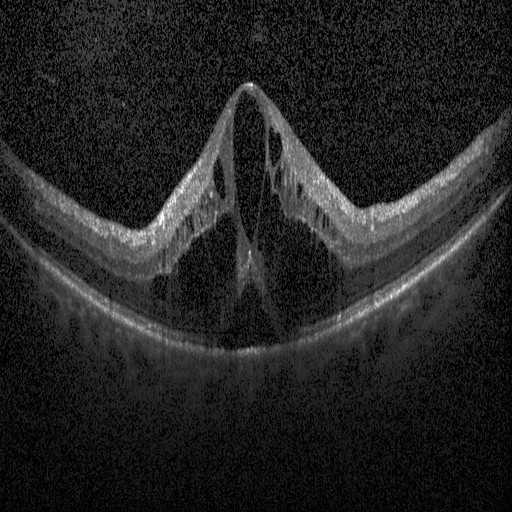 Finding: diabetic macular edema.